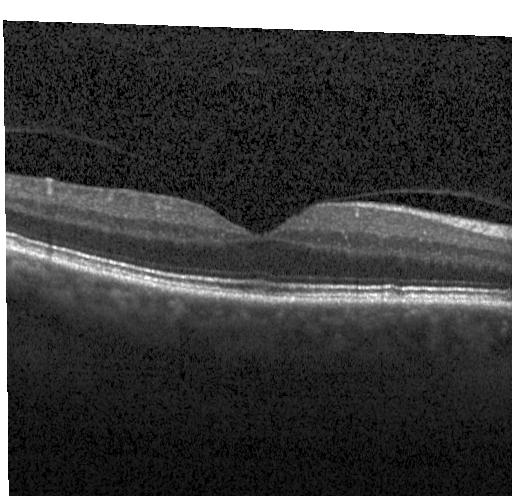

Horizontal scan through the fovea; SD-OCT; retinal OCT B-scan; Heidelberg Spectralis OCT system — The scan shows no CNV, no DME, and no drusen.